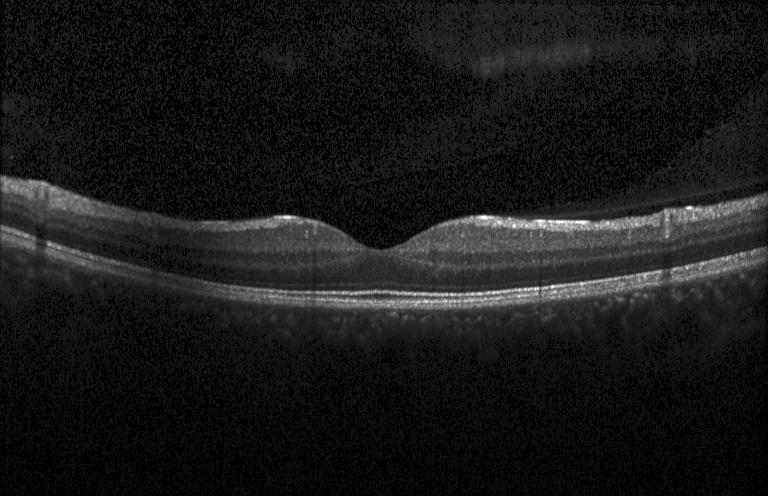

OCT scan showing no choroidal neovascularization, no diabetic macular edema, and no drusen.